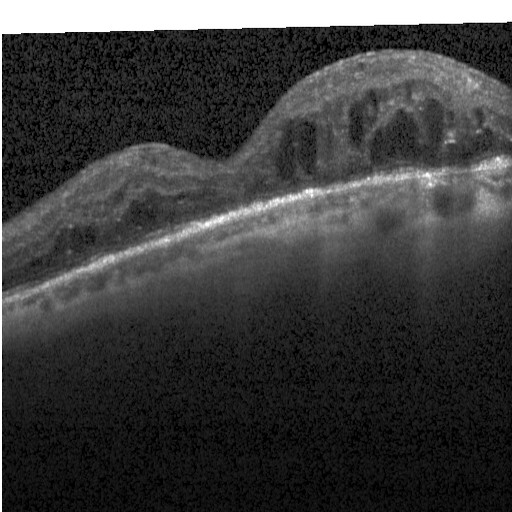
Acquired on a Heidelberg Spectralis, retinal OCT cross-section, through the macula, spectral-domain optical coherence tomography
Macular OCT: DME.